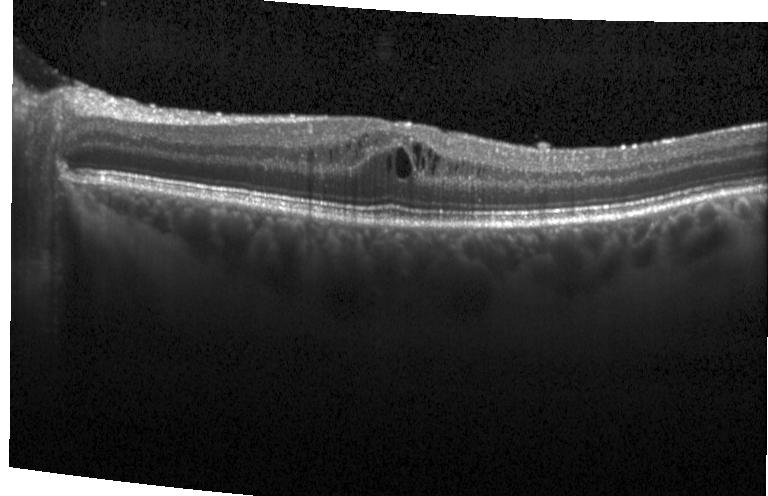

Retinal OCT cross-section; through the macula; Heidelberg Spectralis; spectral-domain optical coherence tomography.
Impression: diabetic macular edema.